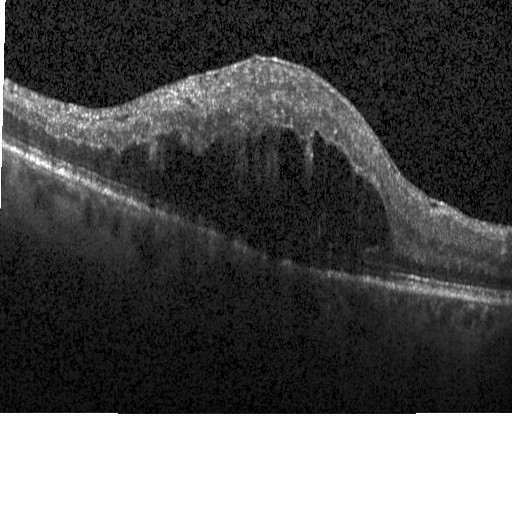

This B-scan demonstrates DME.